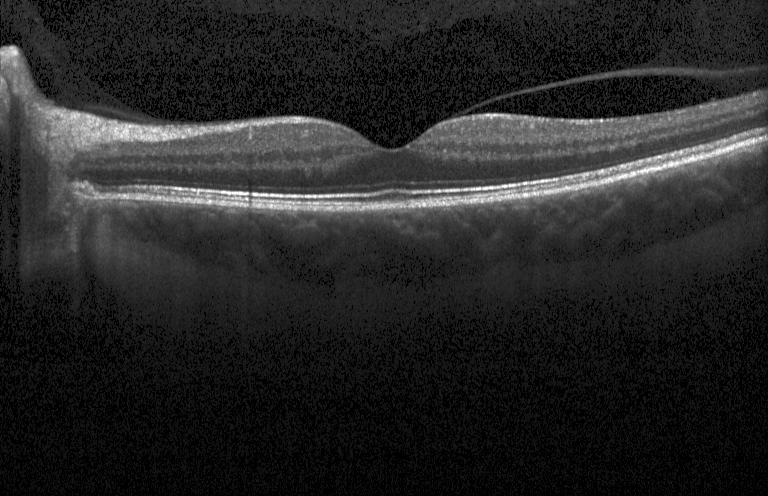

Diagnosis: no choroidal neovascularization, no diabetic macular edema, and no drusen.